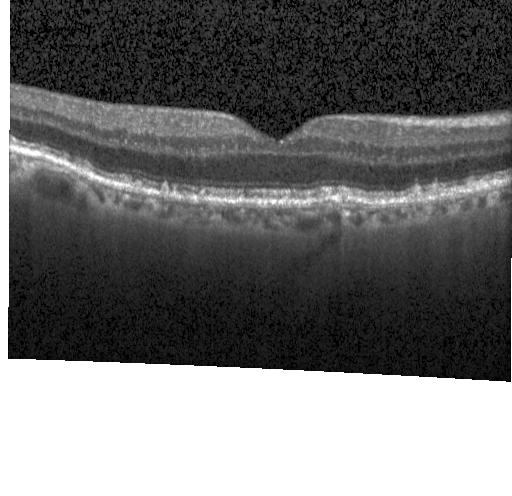 Finding: multiple drusen.